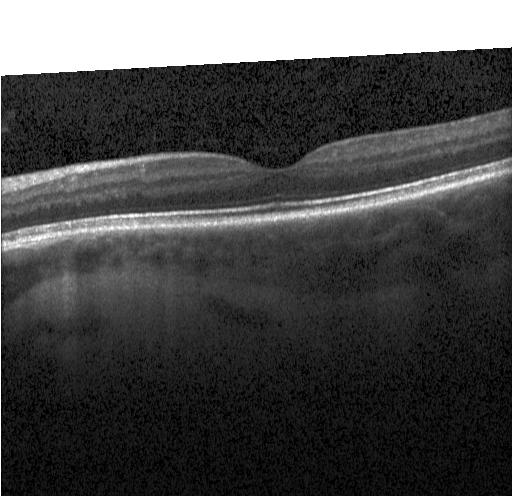
Optical coherence tomography scan. Spectral-domain OCT. Instrument: Heidelberg Spectralis. Horizontal scan through the fovea — OCT finding: no evidence of choroidal neovascularization, diabetic macular edema, or drusen.